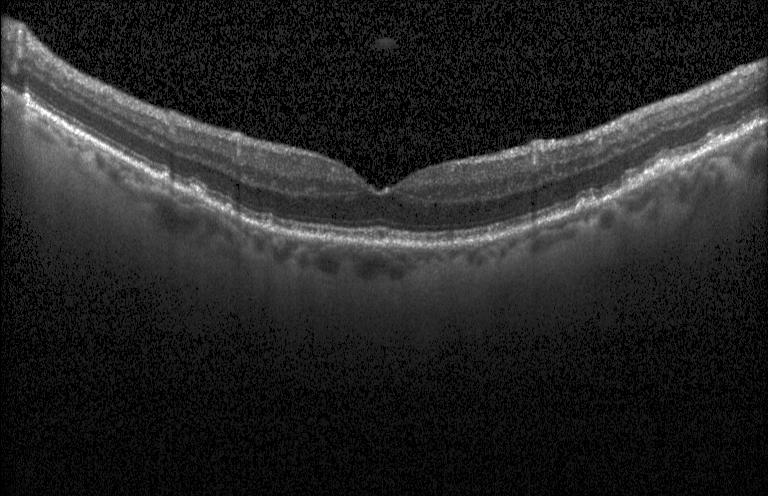

Optical coherence tomography scan — Dx: drusen.